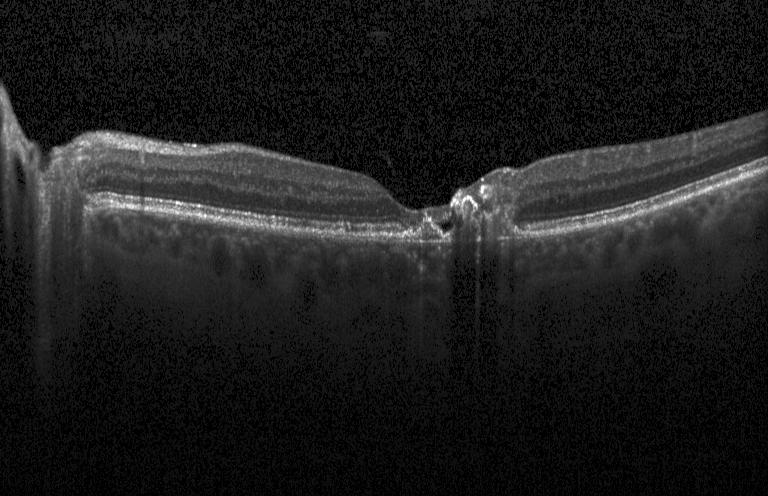 OCT line scan
The scan shows choroidal neovascularization (CNV).